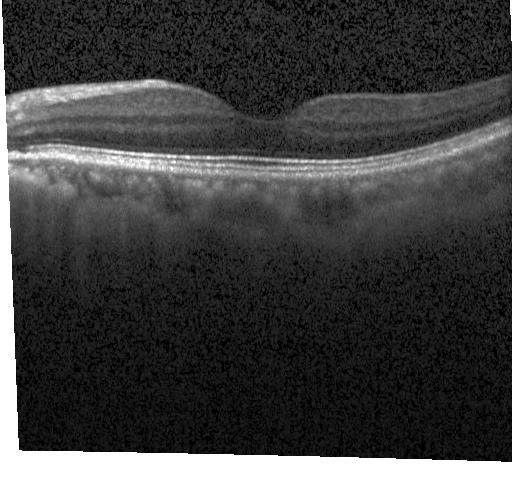

OCT B-scan · Heidelberg Spectralis
Neither CNV, DME, nor drusen.